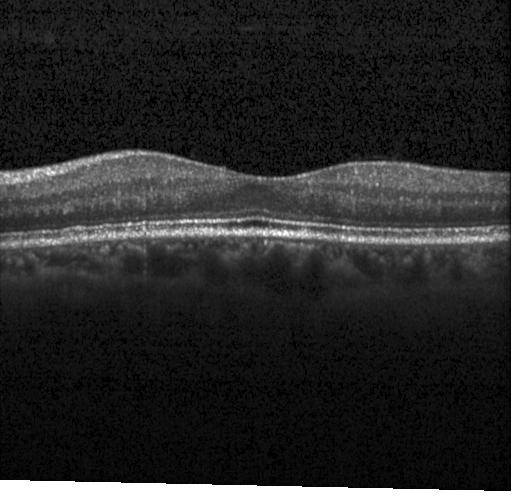

Retinal OCT cross-section showing no choroidal neovascularization, no diabetic macular edema, and no drusen.